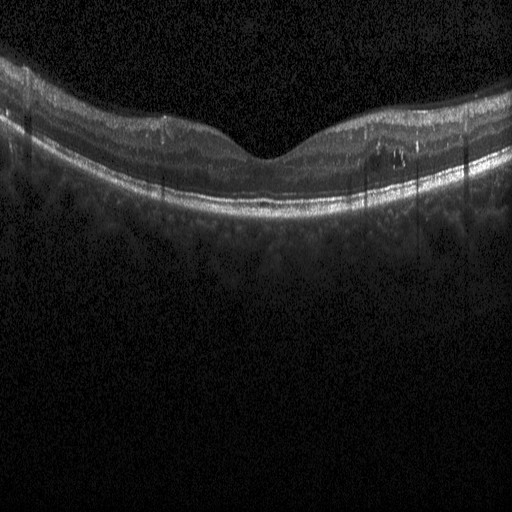 SD-OCT. OCT line scan. Diabetic macular edema.